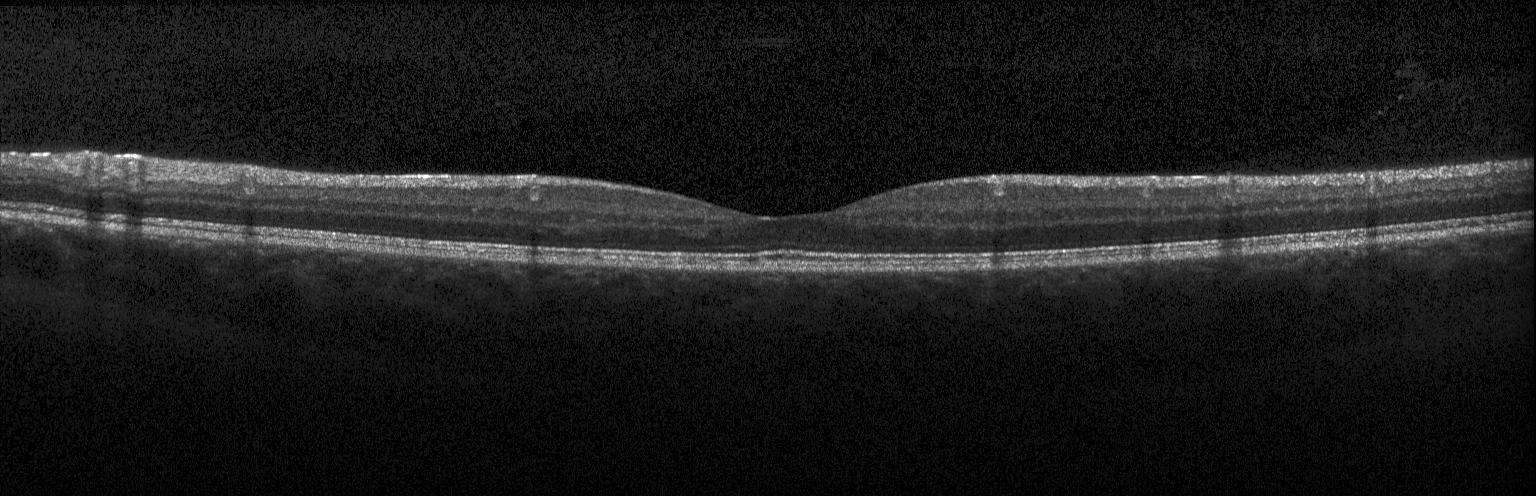

Diagnosis: neither choroidal neovascularization, diabetic macular edema, nor drusen.